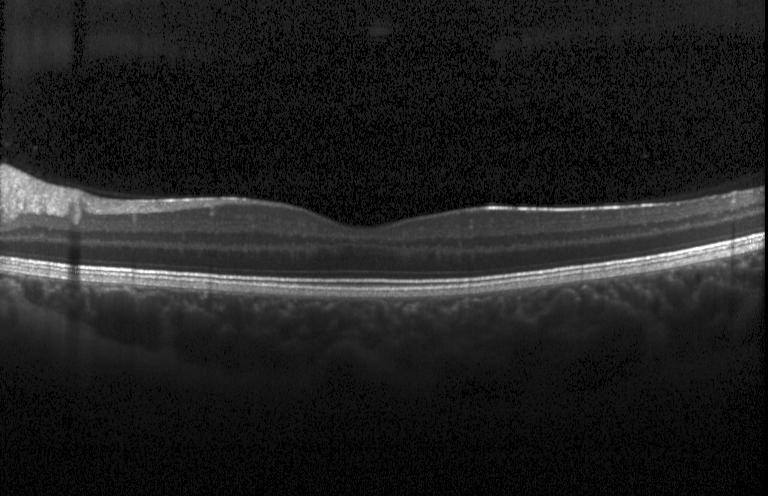
This B-scan demonstrates no evidence of choroidal neovascularization, diabetic macular edema, or drusen.